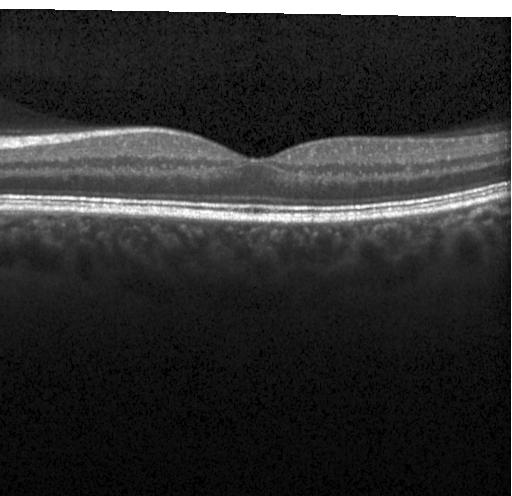 SD-OCT; acquired on a Heidelberg Spectralis; OCT B-scan; fovea-centered.
OCT finding: no choroidal neovascularization, no diabetic macular edema, and no drusen.